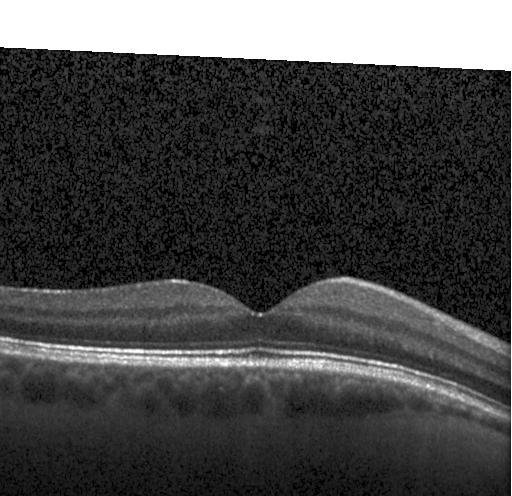 Optical coherence tomography scan.
Impression: no choroidal neovascularization, diabetic macular edema, or drusen.